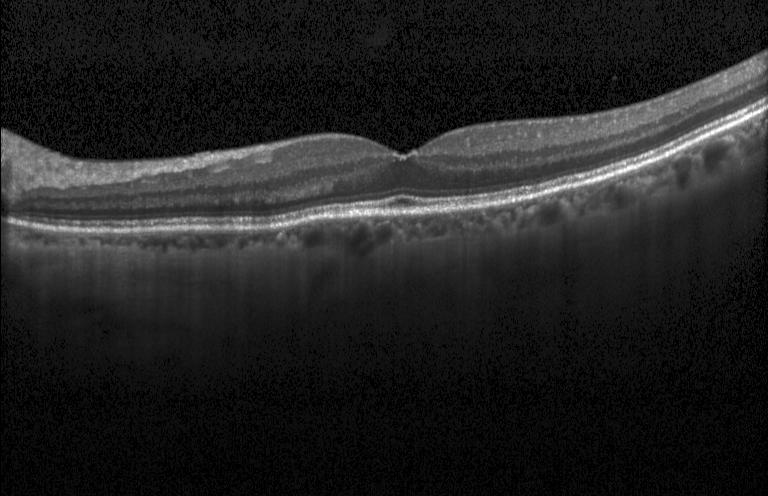

This B-scan demonstrates no CNV, DME, or drusen.